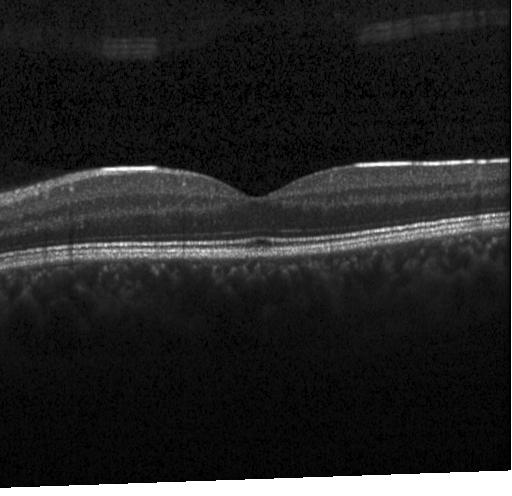

Diagnosis: no choroidal neovascularization, diabetic macular edema, or drusen.